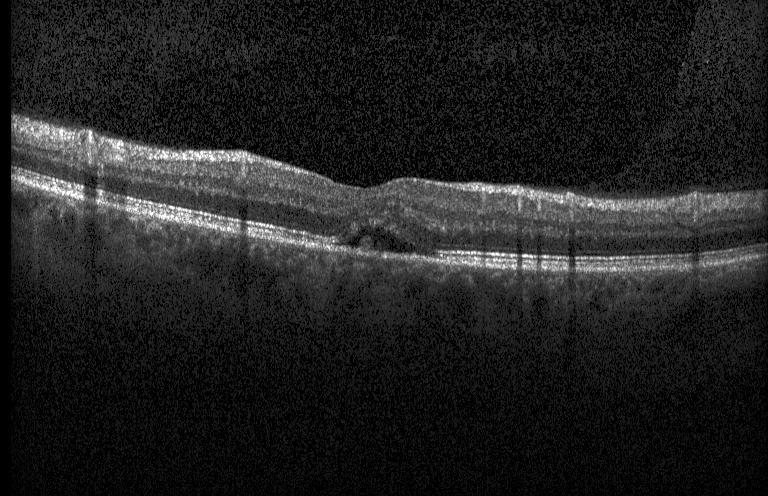
Dx: a choroidal neovascular membrane.